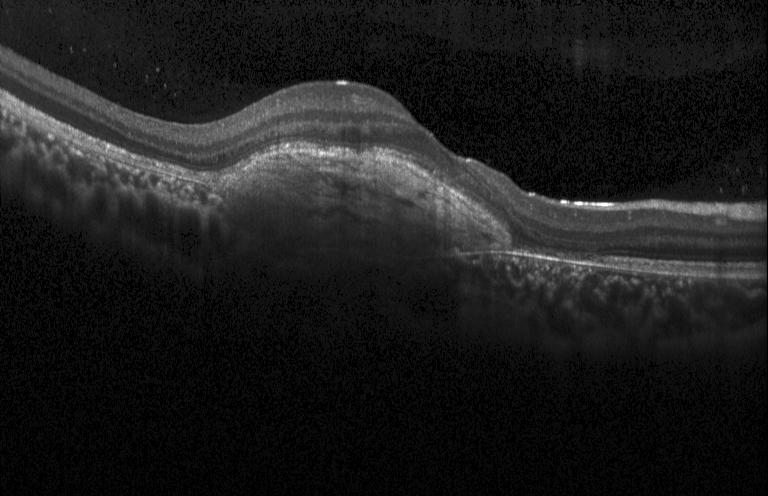

OCT B-scan; spectral-domain optical coherence tomography; Heidelberg Spectralis
A choroidal neovascular membrane.